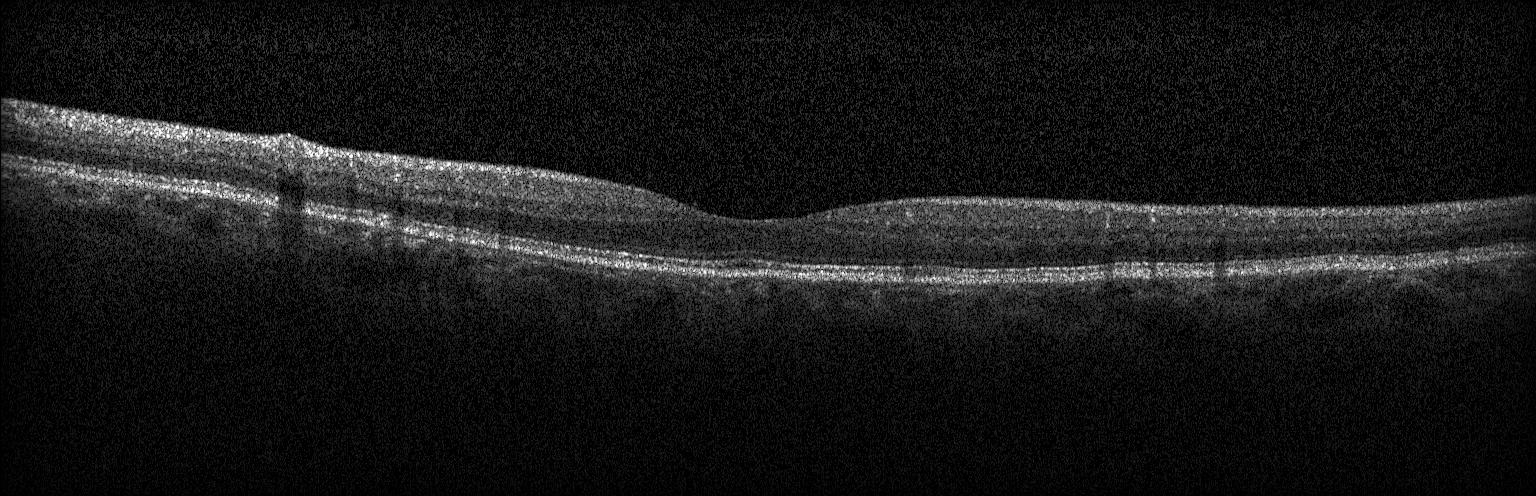
OCT line scan. Heidelberg Spectralis.
The scan shows no choroidal neovascularization, no diabetic macular edema, and no drusen.